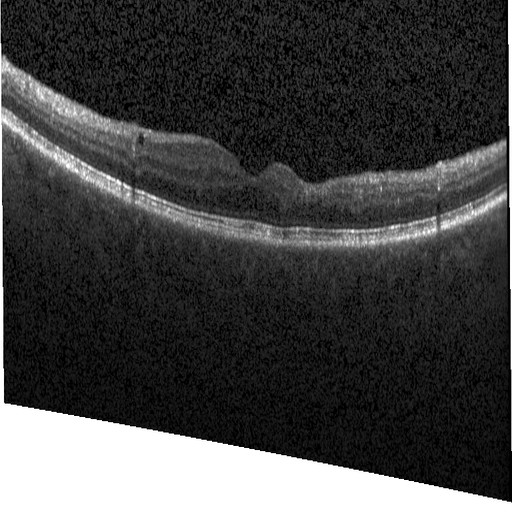

Macular scan; retinal OCT cross-section; instrument: Heidelberg Spectralis; spectral-domain OCT
Impression: DME.